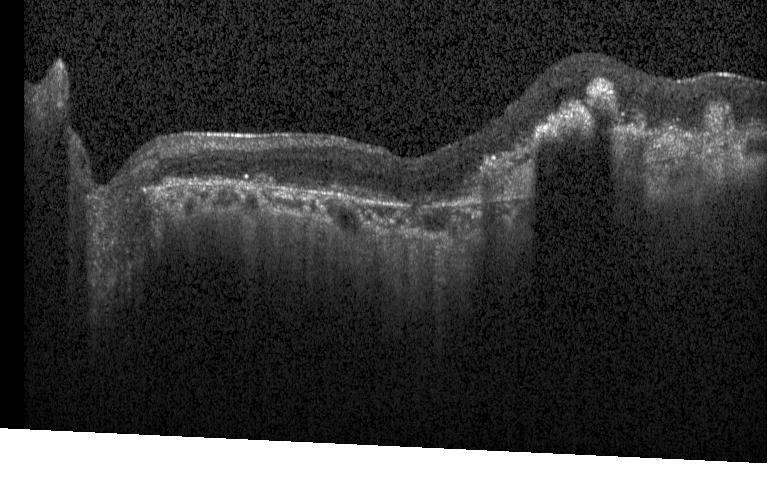

Macular OCT demonstrating a choroidal neovascular membrane.